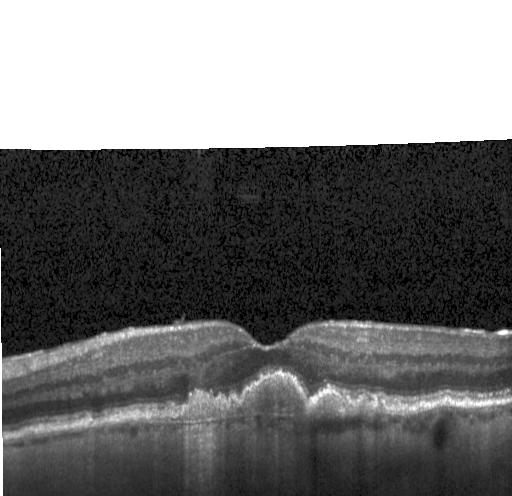
Macular scan · spectral-domain OCT · retinal OCT cross-section · Heidelberg Spectralis OCT system — Diagnosis: a choroidal neovascular membrane.